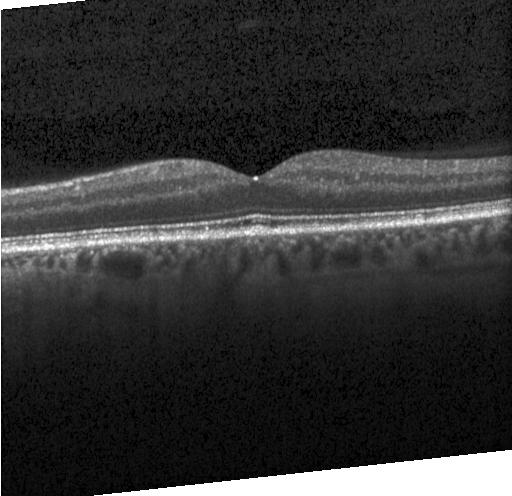 Heidelberg Spectralis · optical coherence tomography scan · fovea-centered. Diagnosis: no CNV, DME, or drusen.